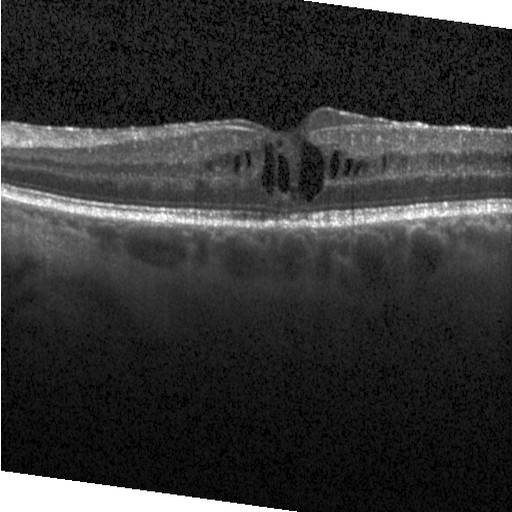

Optical coherence tomography scan — Impression: DME.